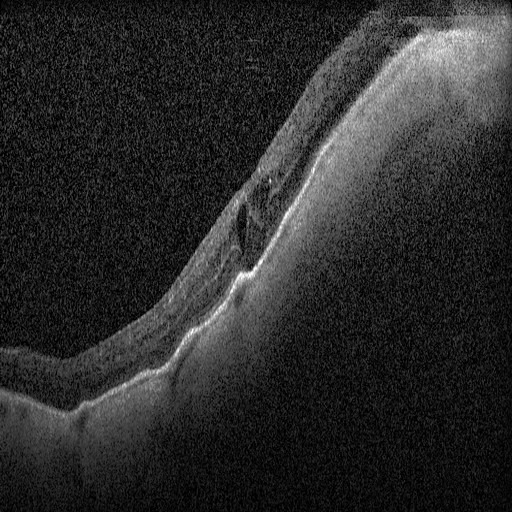
Assessment: diabetic macular edema.